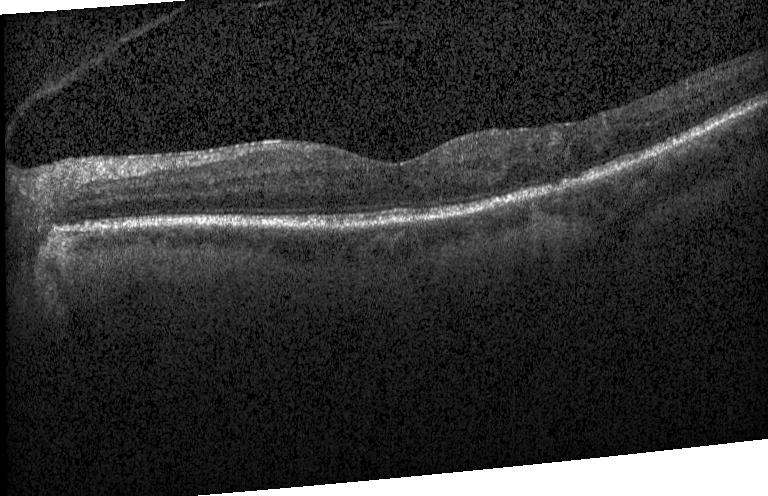 OCT finding: diabetic macular edema (DME).